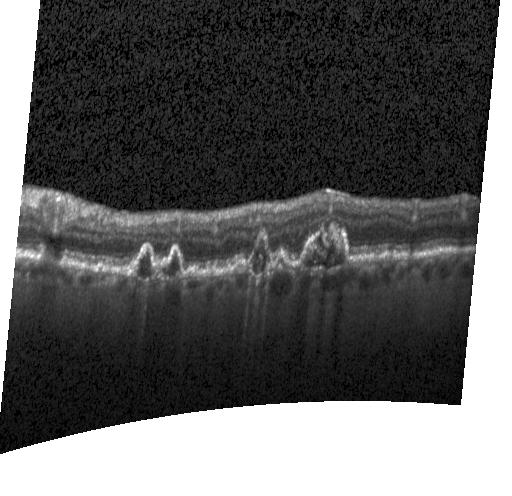 Instrument: Heidelberg Spectralis. Optical coherence tomography scan. Spectral-domain optical coherence tomography.
Finding: choroidal neovascularization (CNV).